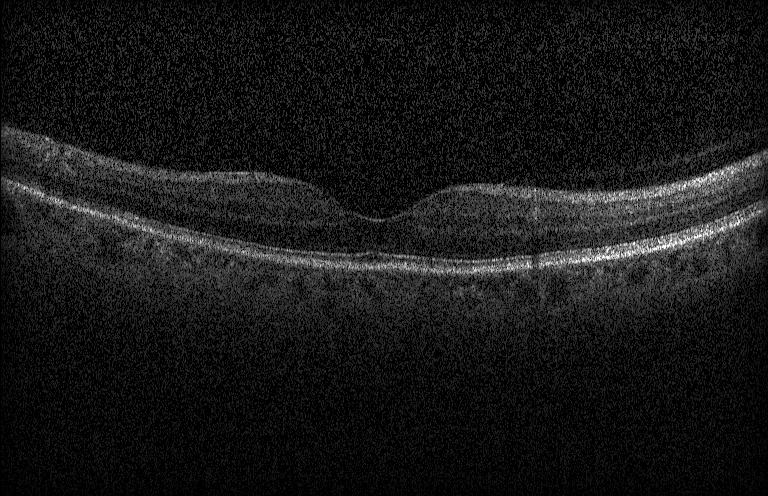
The scan shows neither choroidal neovascularization, diabetic macular edema, nor drusen.